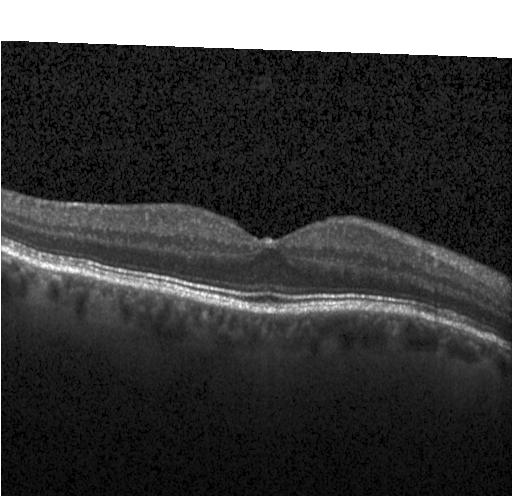
OCT B-scan · acquired on a Heidelberg Spectralis · fovea-centered — Impression: no choroidal neovascularization, no diabetic macular edema, and no drusen.